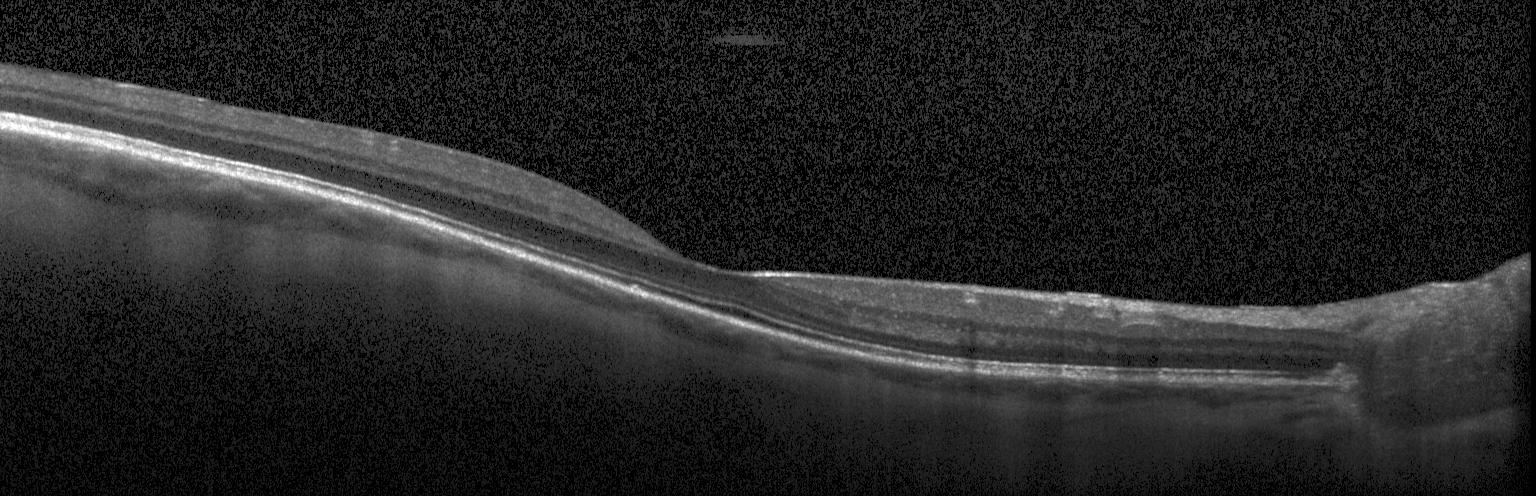
Instrument: Heidelberg Spectralis · through the macula · SD-OCT · optical coherence tomography scan — No evidence of choroidal neovascularization, diabetic macular edema, or drusen.